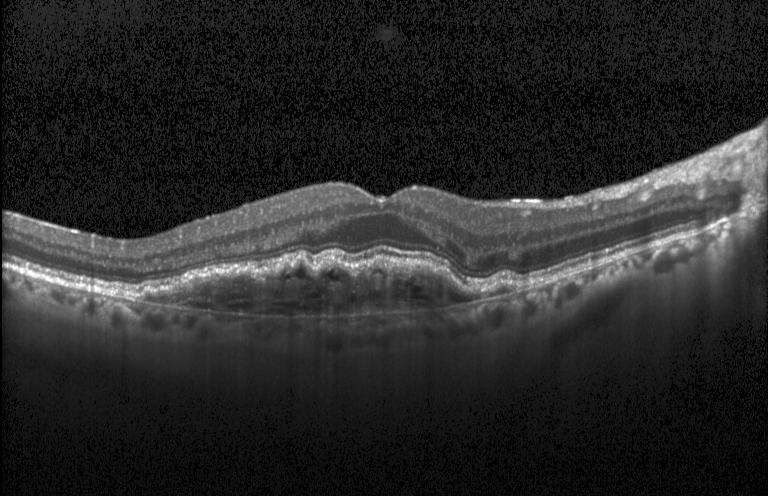

Retinal OCT cross-section — Diagnosis: choroidal neovascularization.